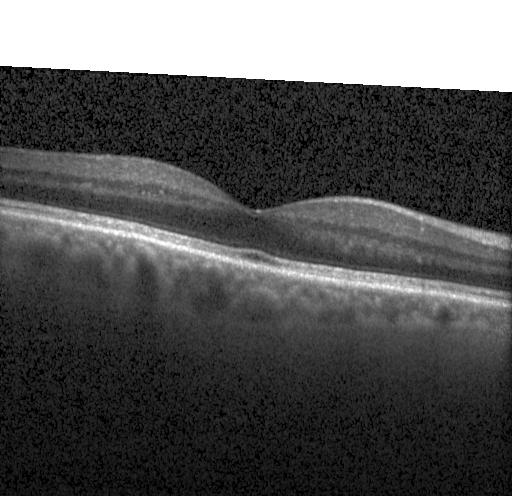
The scan shows no choroidal neovascularization, diabetic macular edema, or drusen.